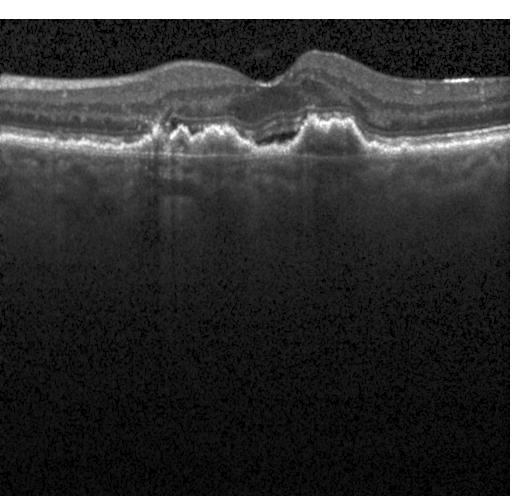
Heidelberg Spectralis. OCT line scan.
OCT finding: a choroidal neovascular membrane.